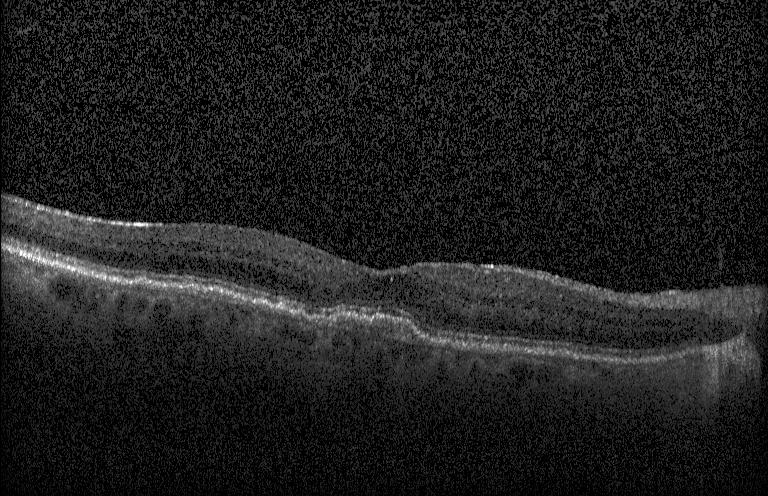 OCT finding: a choroidal neovascular membrane.